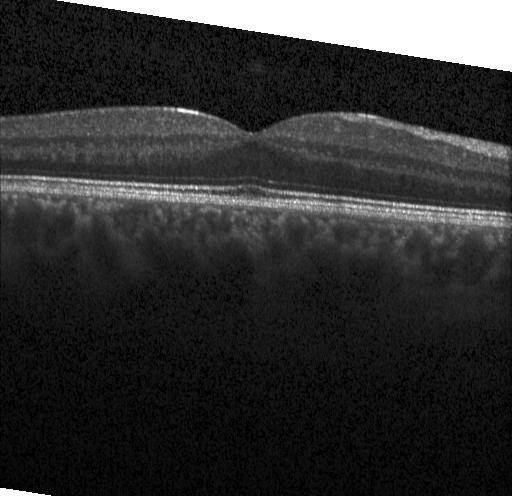 Spectral-domain OCT B-scan: no CNV, no DME, and no drusen.